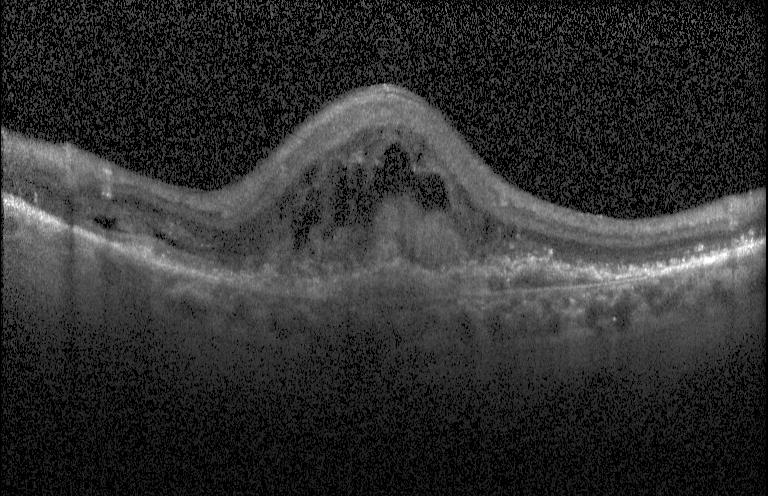
Optical coherence tomography B-scan · acquired on a Heidelberg Spectralis · SD-OCT · fovea-centered. Dx: choroidal neovascularization (CNV).